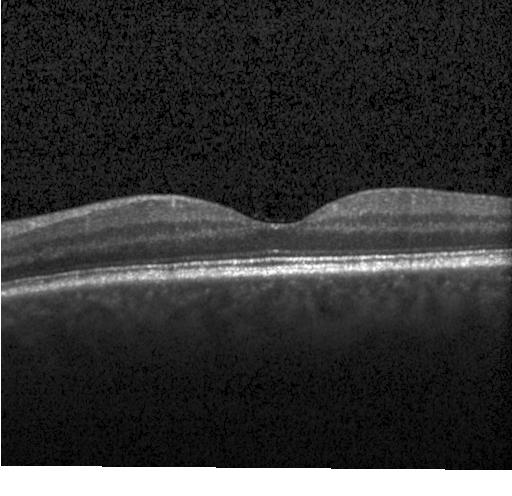

Spectral-domain optical coherence tomography. Optical coherence tomography scan. Fovea-centered
Macular OCT: no CNV, DME, or drusen.